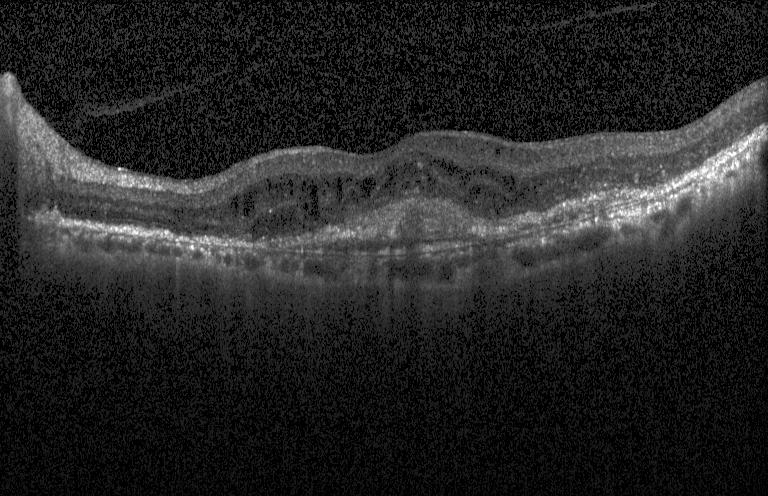
Fovea-centered; instrument: Heidelberg Spectralis; spectral-domain OCT; retinal OCT cross-section.
Diagnosis: choroidal neovascularization.